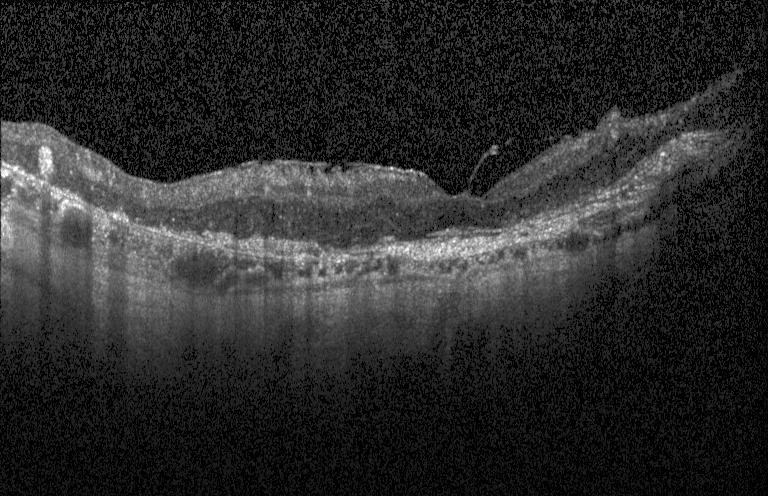
Optical coherence tomography B-scan. Assessment: choroidal neovascularization.